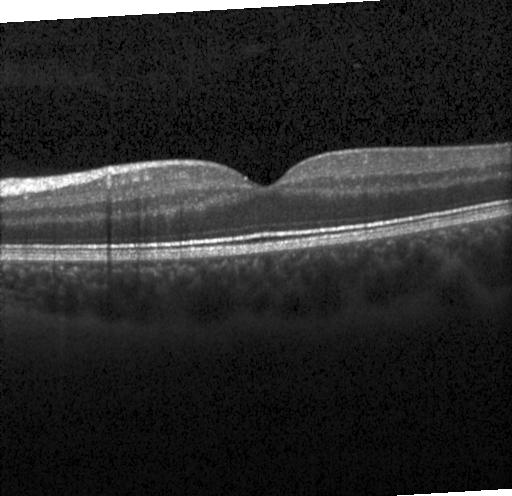 This B-scan demonstrates no choroidal neovascularization, diabetic macular edema, or drusen.